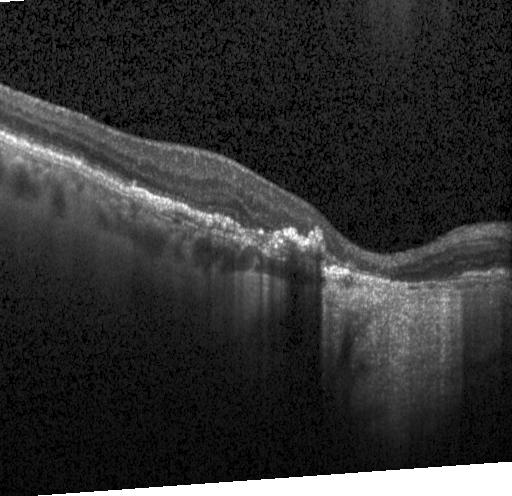

Fovea-centered. Optical coherence tomography B-scan. Heidelberg Spectralis OCT system. Spectral-domain OCT.
Diagnosis: a choroidal neovascular membrane.